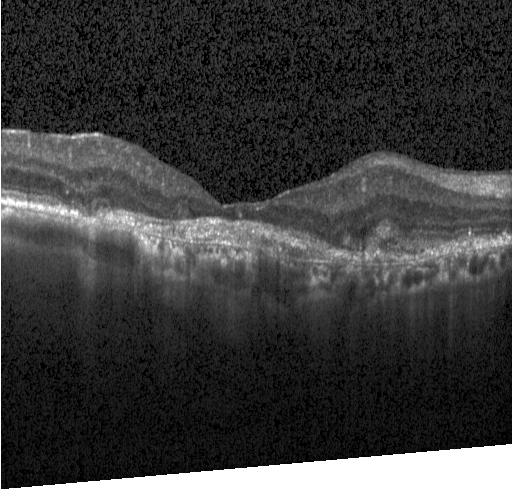
Retinal OCT cross-section · acquired on a Heidelberg Spectralis
Diagnosis: a choroidal neovascular membrane.